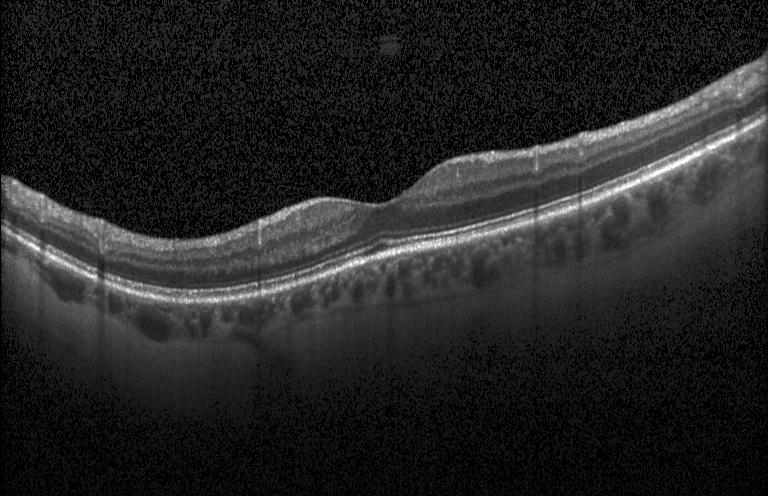 Diagnosis: no choroidal neovascularization, no diabetic macular edema, and no drusen.